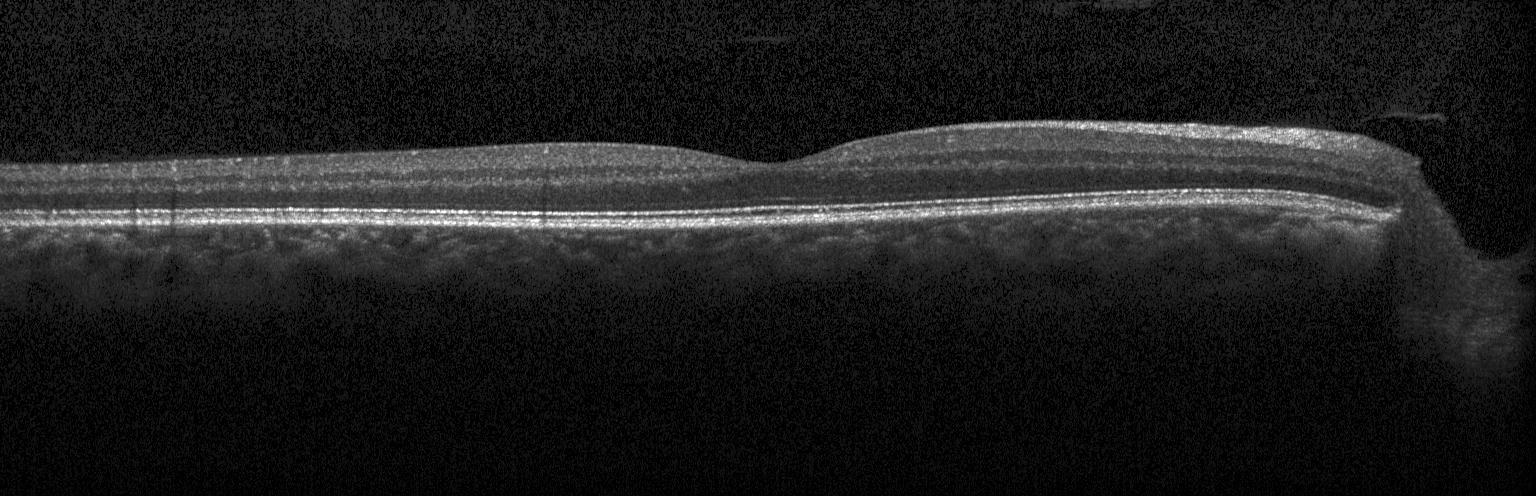
OCT B-scan. This B-scan demonstrates no evidence of CNV, DME, or drusen.